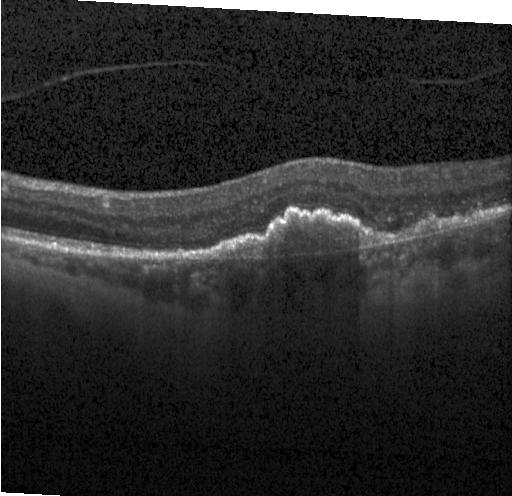
Heidelberg Spectralis; spectral-domain OCT; horizontal scan through the fovea; retinal OCT B-scan.
Diagnosis: choroidal neovascularization (CNV).